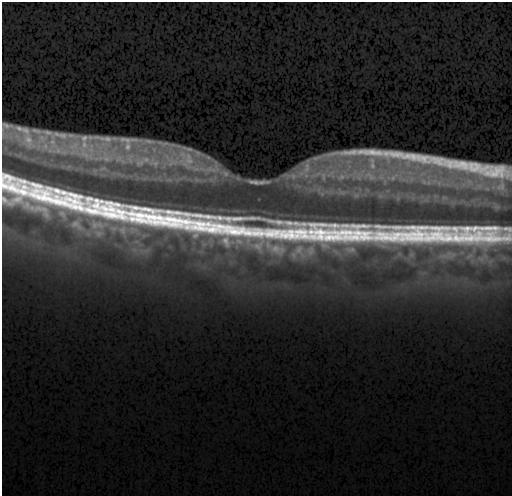

Macular OCT demonstrating no CNV, no DME, and no drusen.